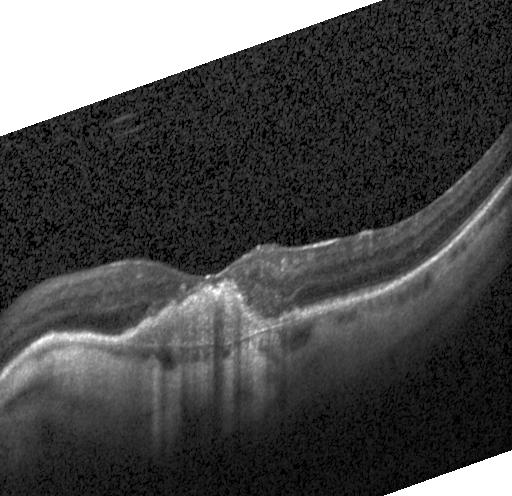

SD-OCT; fovea-centered; acquired on a Heidelberg Spectralis; retinal OCT B-scan. Diagnosis: CNV.